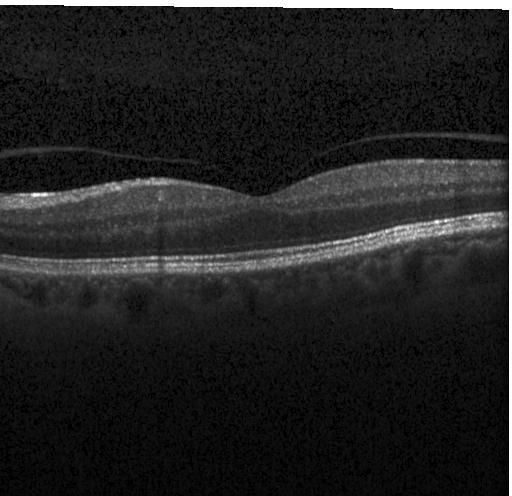

Retinal OCT cross-section
Impression: no CNV, no DME, and no drusen.